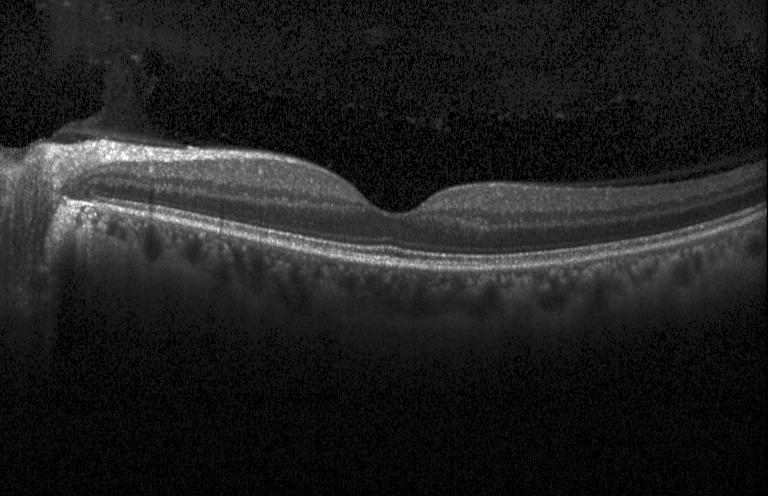

Horizontal scan through the fovea · instrument: Heidelberg Spectralis · optical coherence tomography scan · spectral-domain optical coherence tomography
Impression: no choroidal neovascularization, no diabetic macular edema, and no drusen.